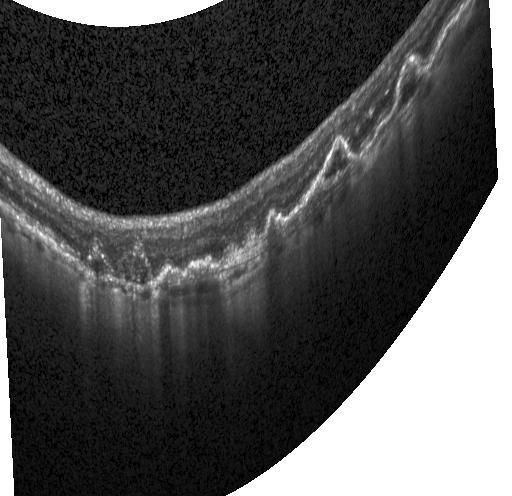
Horizontal scan through the fovea. Optical coherence tomography scan. Instrument: Heidelberg Spectralis. Spectral-domain optical coherence tomography
CNV.